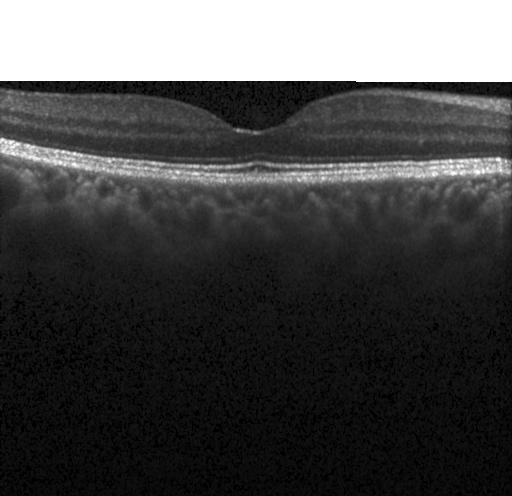
Retinal OCT cross-section.
Dx: no evidence of choroidal neovascularization, diabetic macular edema, or drusen.